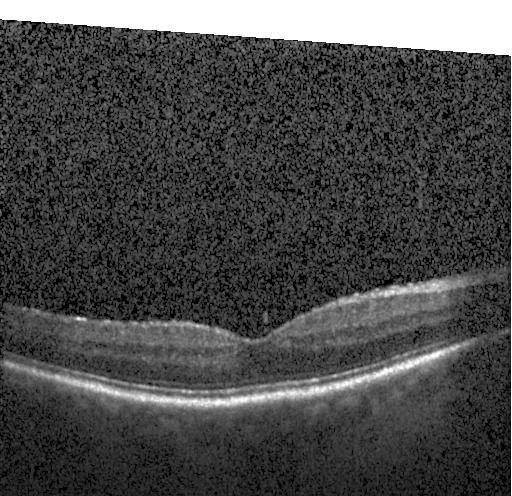
The scan shows no evidence of CNV, DME, or drusen.